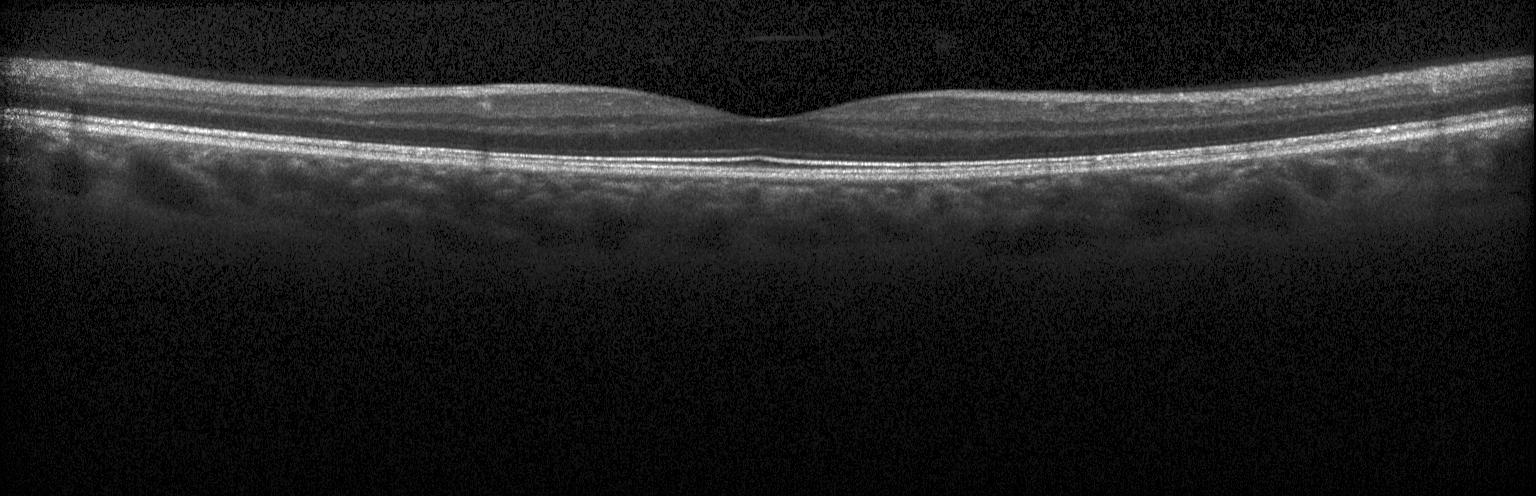
Spectral-domain optical coherence tomography. Retinal OCT B-scan. Instrument: Heidelberg Spectralis. Macular scan.
Impression: neither choroidal neovascularization, diabetic macular edema, nor drusen.